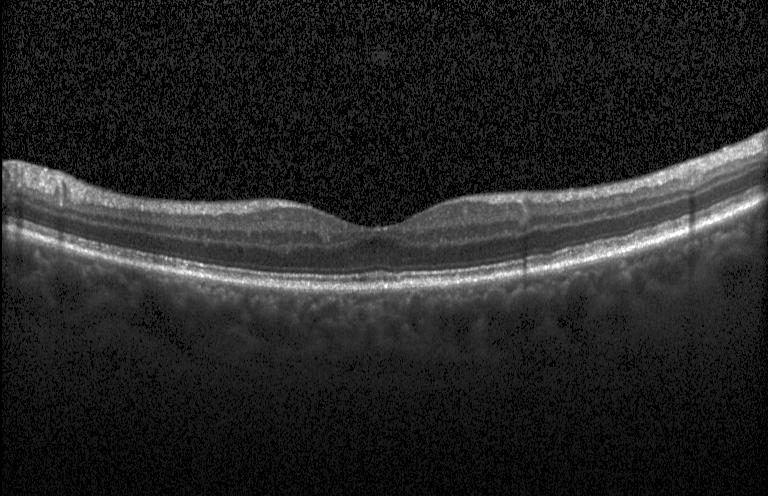 Retinal OCT B-scan. Fovea-centered. The scan shows no choroidal neovascularization, diabetic macular edema, or drusen.